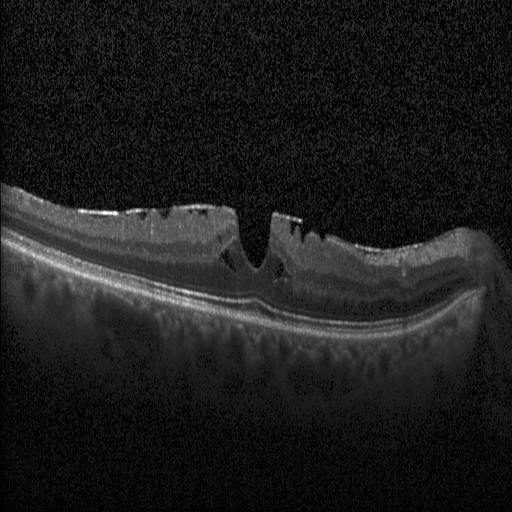
Optical coherence tomography B-scan
Assessment: diabetic macular edema.